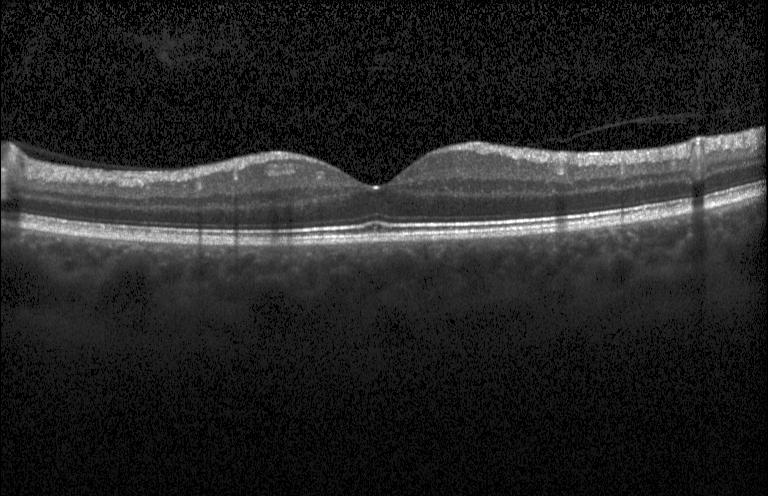

Optical coherence tomography B-scan — Macular OCT: no choroidal neovascularization, diabetic macular edema, or drusen.